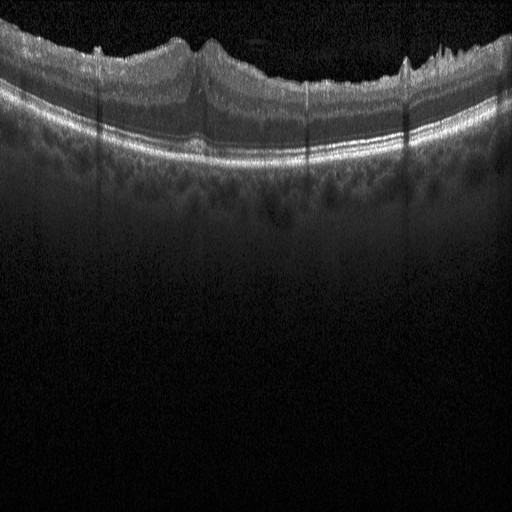
Spectral-domain OCT B-scan: diabetic macular edema (DME).